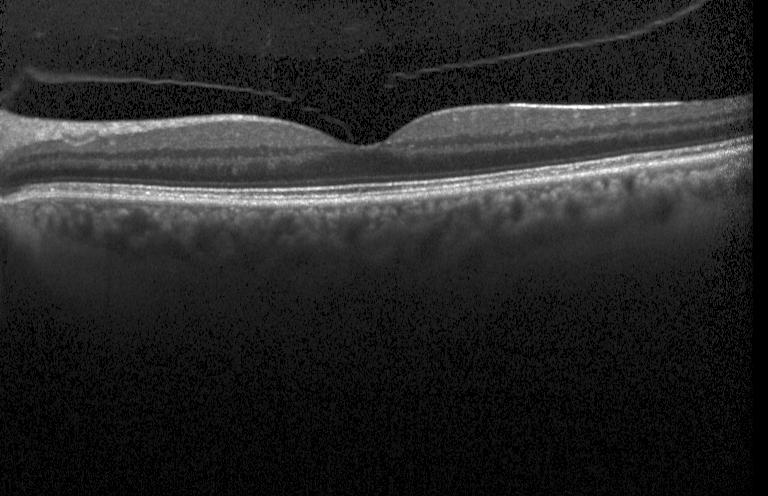

Spectral-domain OCT. Fovea-centered. OCT line scan. Heidelberg Spectralis OCT system — Diagnosis: no evidence of CNV, DME, or drusen.